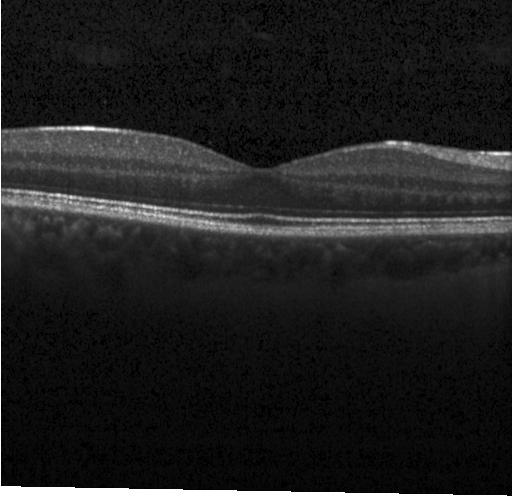 This B-scan demonstrates no evidence of choroidal neovascularization, diabetic macular edema, or drusen.